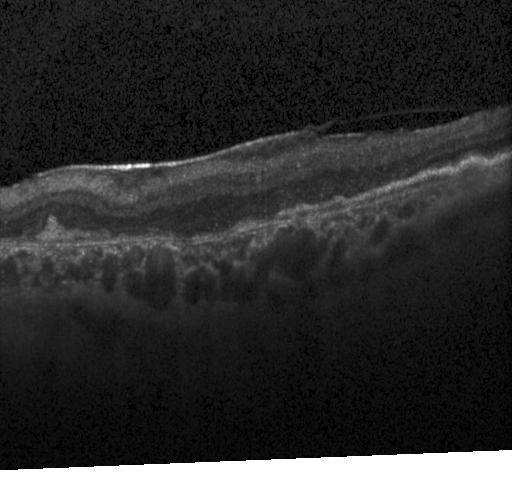
Impression: CNV.